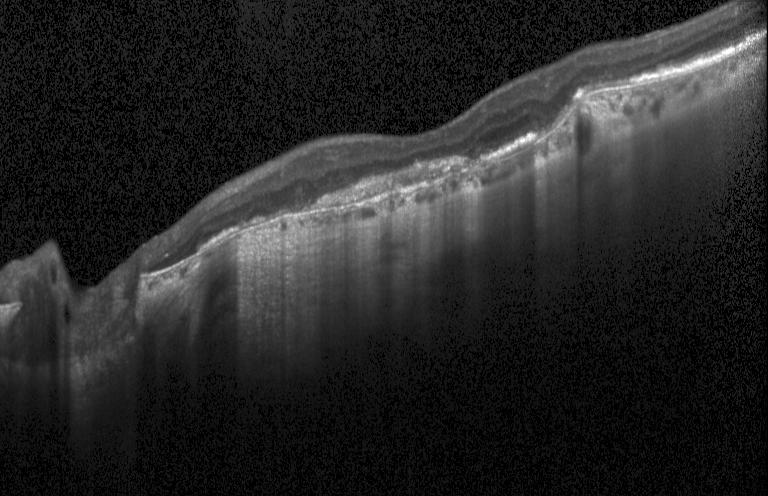
Spectral-domain OCT B-scan: CNV.